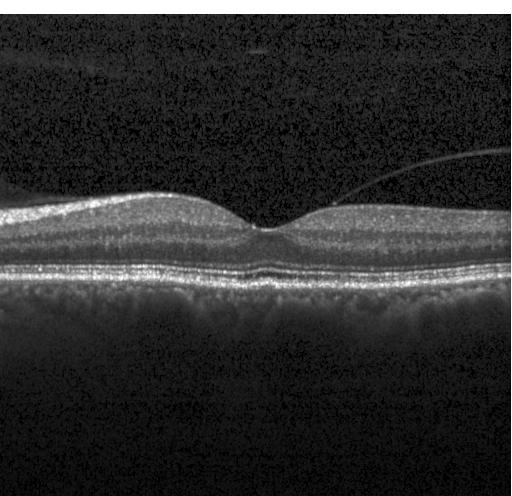

Assessment: no evidence of choroidal neovascularization, diabetic macular edema, or drusen.